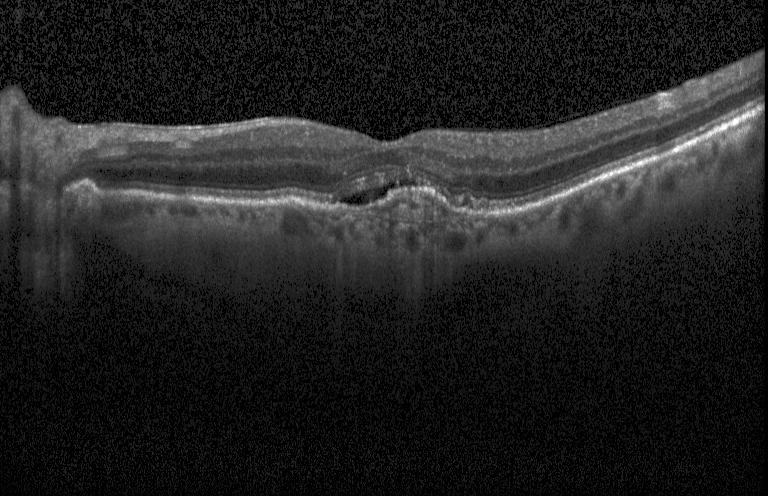 Fovea-centered, acquired on a Heidelberg Spectralis, SD-OCT, retinal OCT cross-section.
Assessment: a choroidal neovascular membrane.